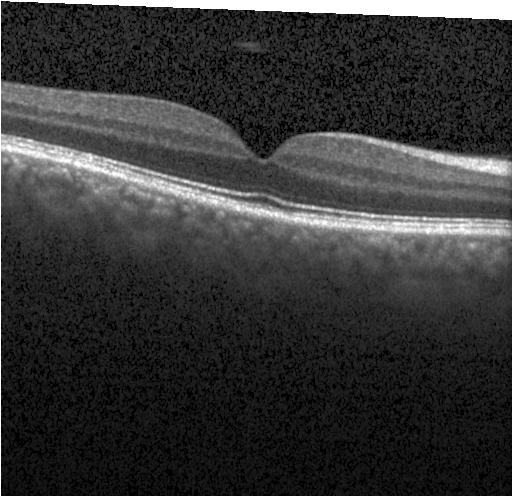
Macular OCT: no choroidal neovascularization, no diabetic macular edema, and no drusen.